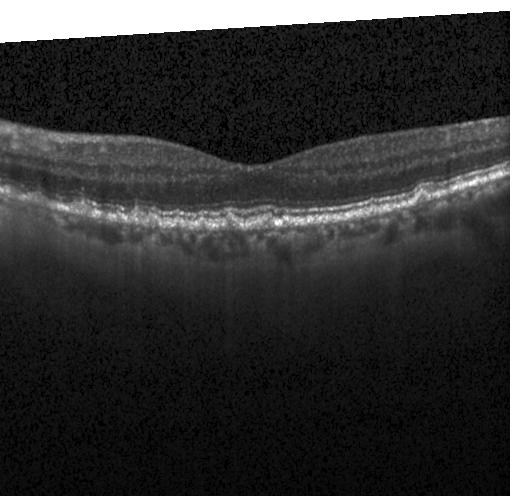
Diagnosis: multiple drusen.